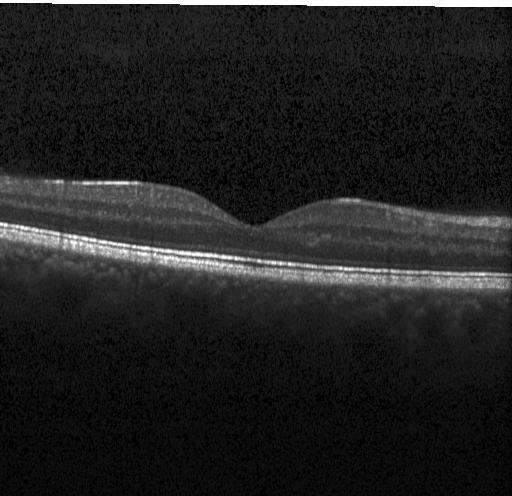
Spectral-domain optical coherence tomography, fovea-centered, optical coherence tomography scan, Heidelberg Spectralis OCT system
Dx: no CNV, DME, or drusen.